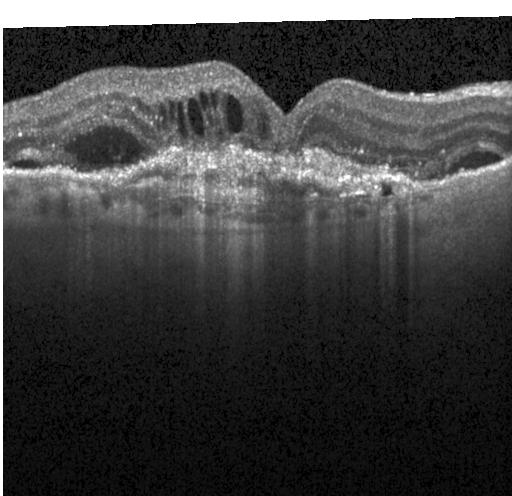

Optical coherence tomography scan, macular scan — Dx: CNV.